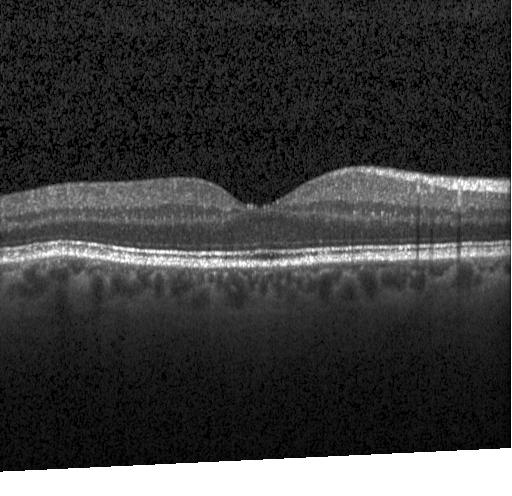

OCT B-scan, spectral-domain OCT, centered on the fovea
Diagnosis: no choroidal neovascularization, diabetic macular edema, or drusen.